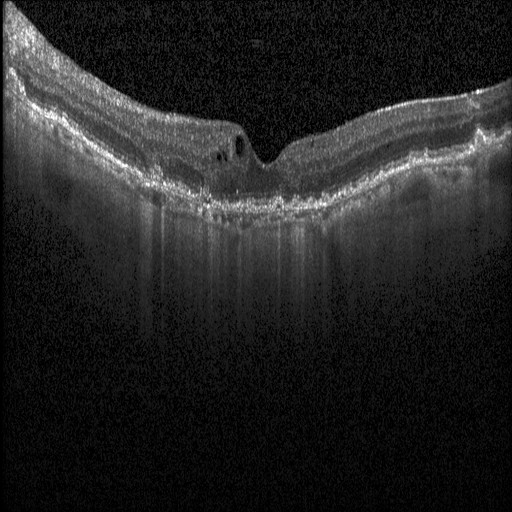 Retinal OCT cross-section showing diabetic macular edema (DME).